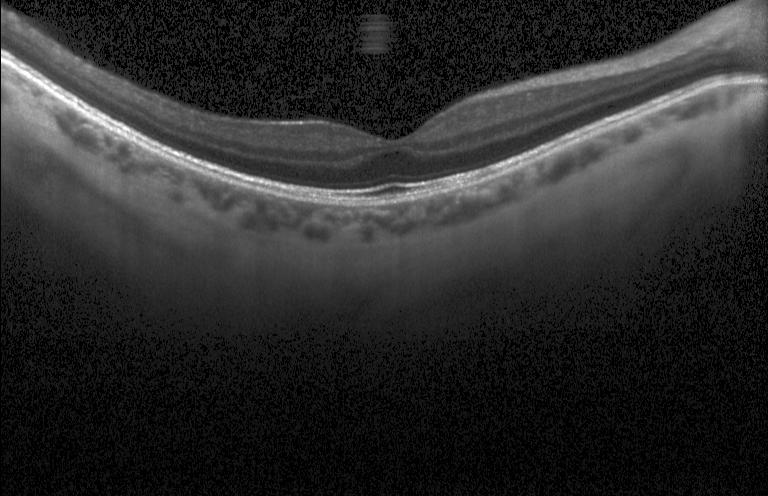

Instrument: Heidelberg Spectralis. Retinal OCT B-scan
Assessment: no evidence of choroidal neovascularization, diabetic macular edema, or drusen.